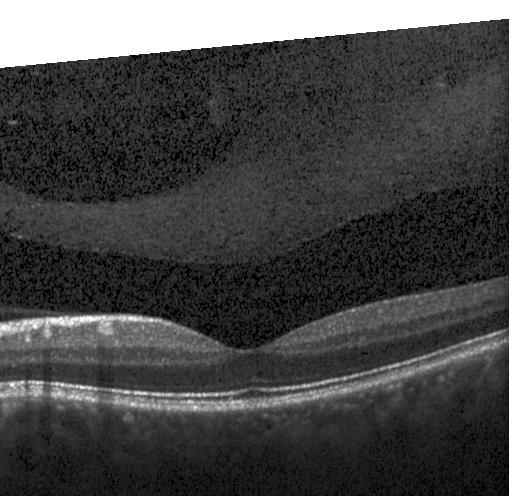 Assessment: no choroidal neovascularization, no diabetic macular edema, and no drusen.